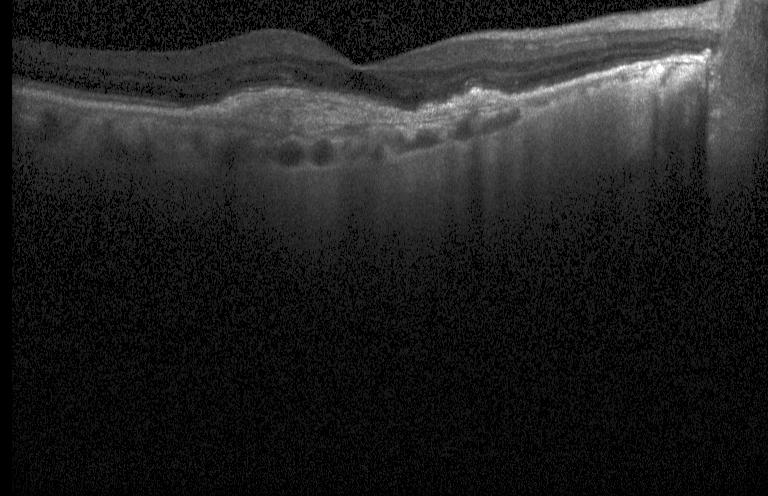
Diagnosis: a choroidal neovascular membrane.